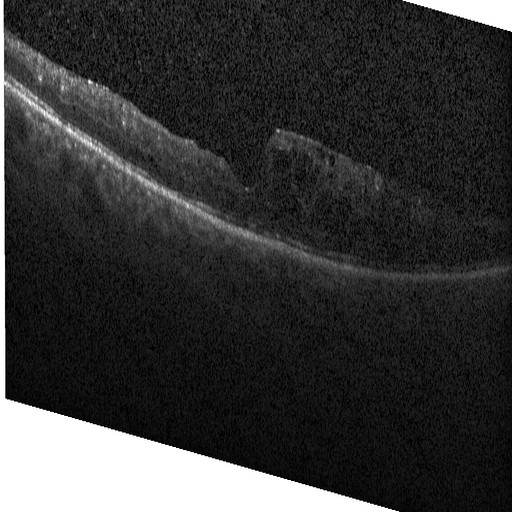

This B-scan demonstrates diabetic macular edema (DME).